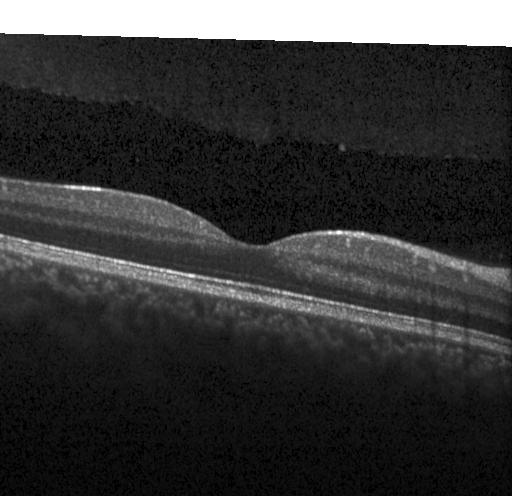
Spectral-domain optical coherence tomography; OCT line scan
Finding: neither CNV, DME, nor drusen.